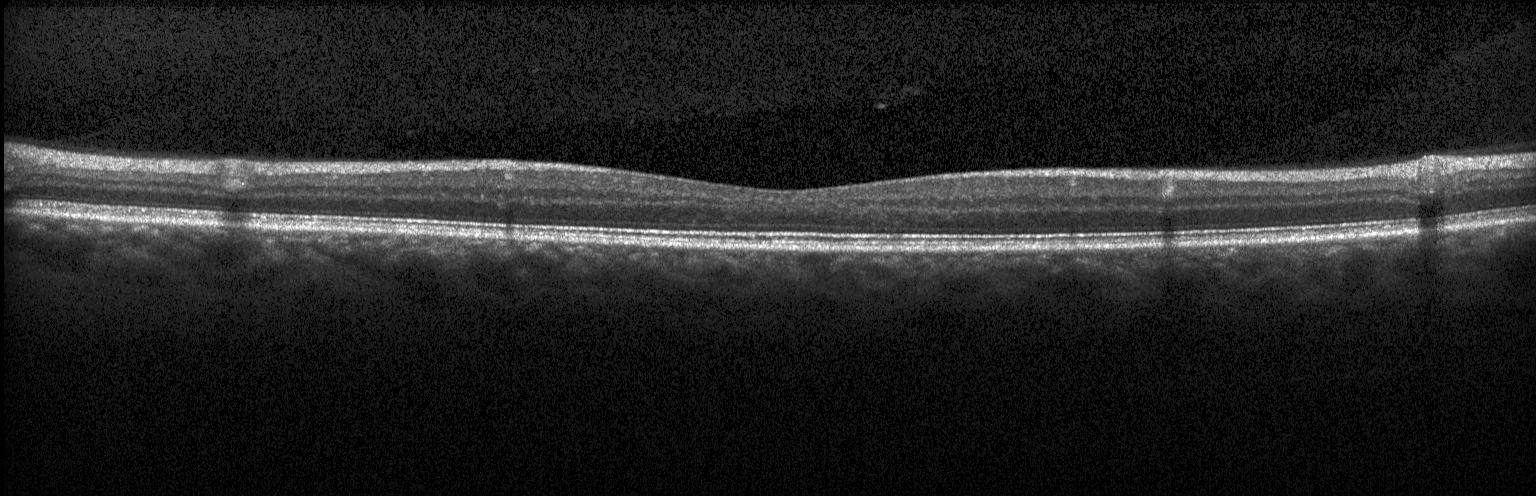

Spectral-domain optical coherence tomography. Instrument: Heidelberg Spectralis. Retinal OCT B-scan. No choroidal neovascularization, no diabetic macular edema, and no drusen.